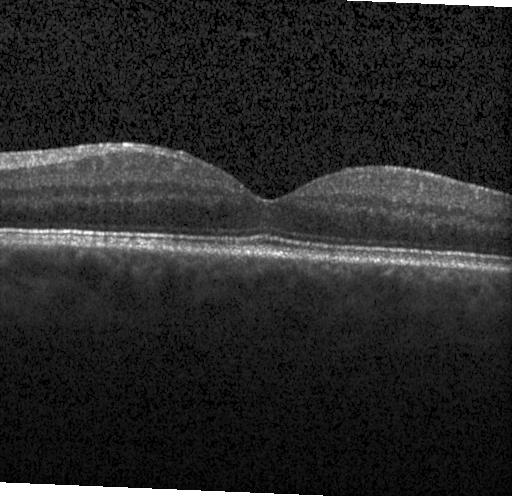 Retinal OCT cross-section showing no choroidal neovascularization, no diabetic macular edema, and no drusen.